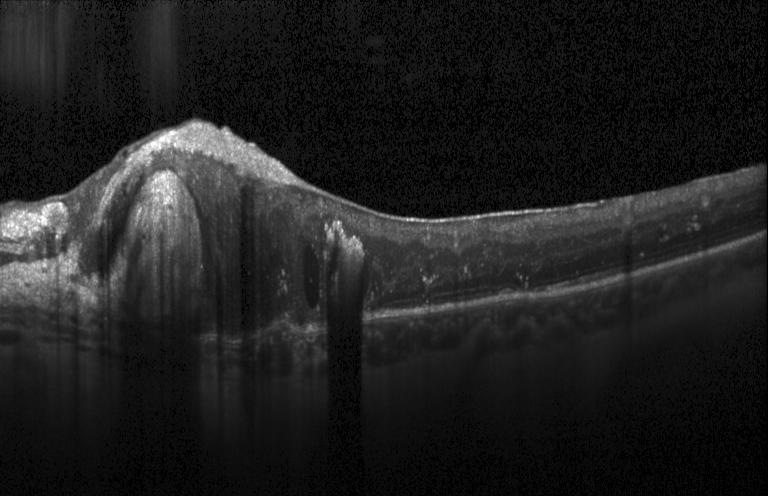 Heidelberg Spectralis · centered on the fovea · optical coherence tomography B-scan · SD-OCT
The scan shows choroidal neovascularization.